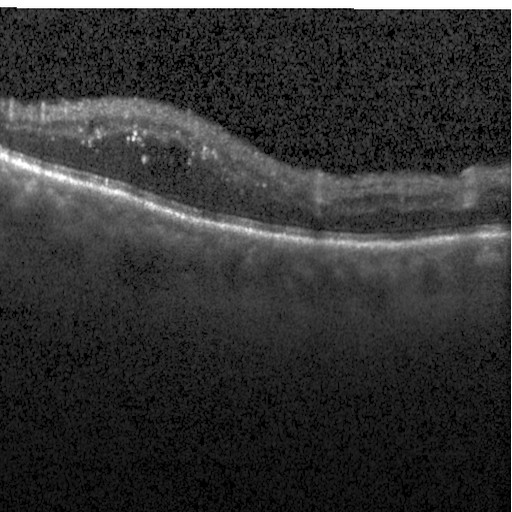 Retinal OCT cross-section. Macular scan. Spectral-domain optical coherence tomography. Acquired on a Heidelberg Spectralis
Assessment: DME.